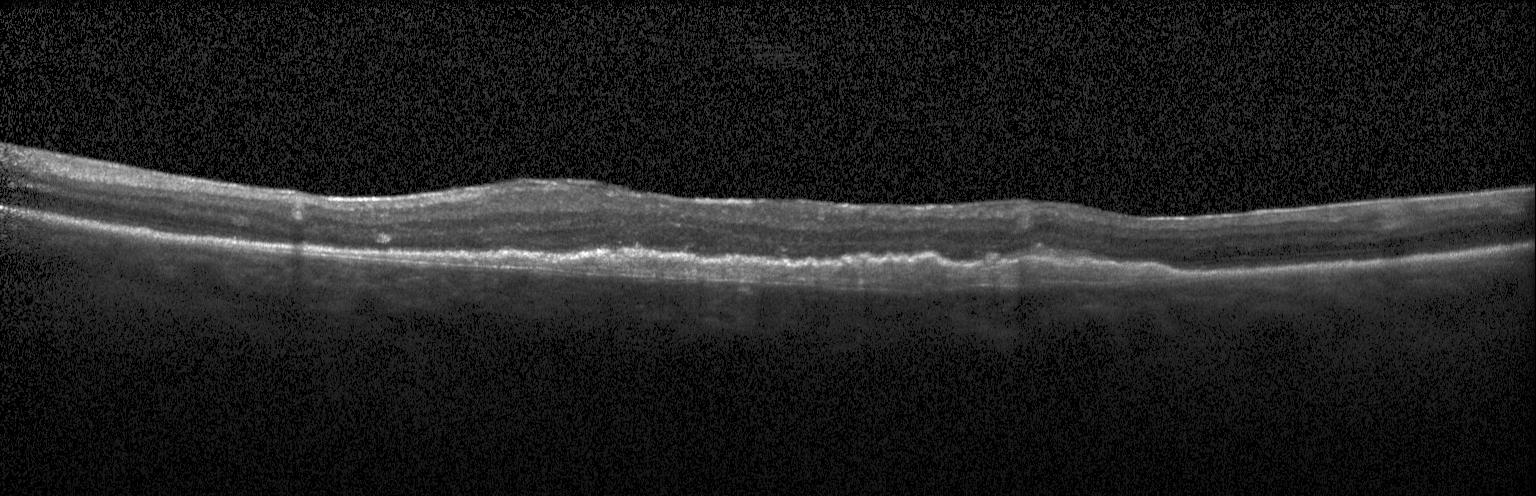

CNV.